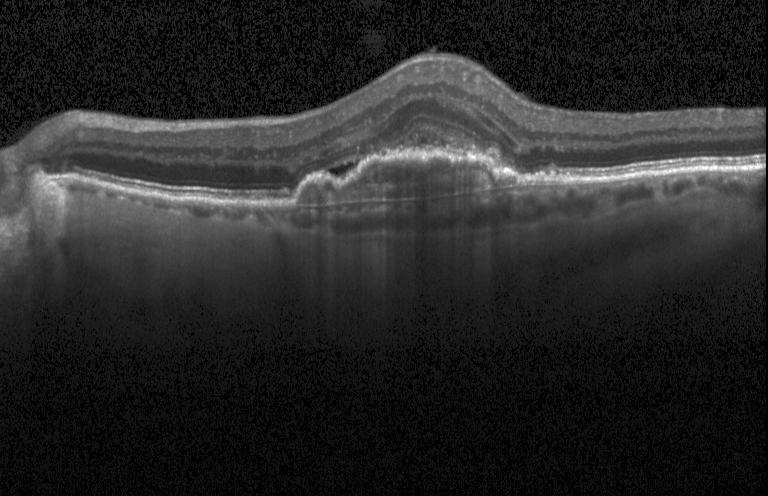

OCT B-scan showing a choroidal neovascular membrane.